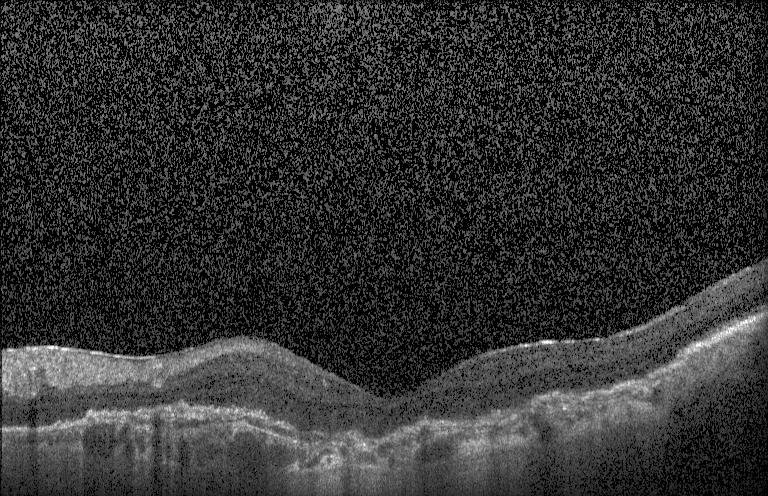 Spectral-domain OCT; horizontal scan through the fovea; OCT B-scan
This B-scan demonstrates choroidal neovascularization.